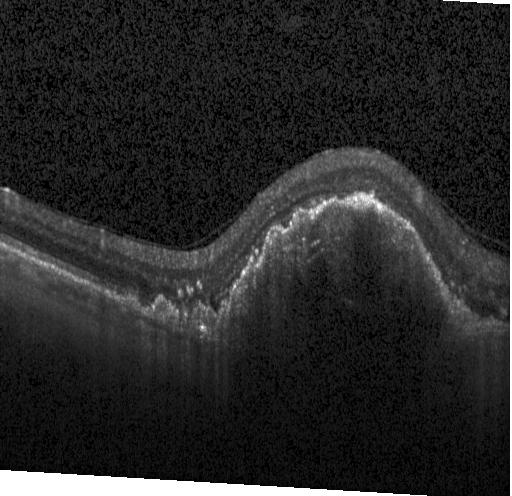 OCT line scan. This B-scan demonstrates CNV.